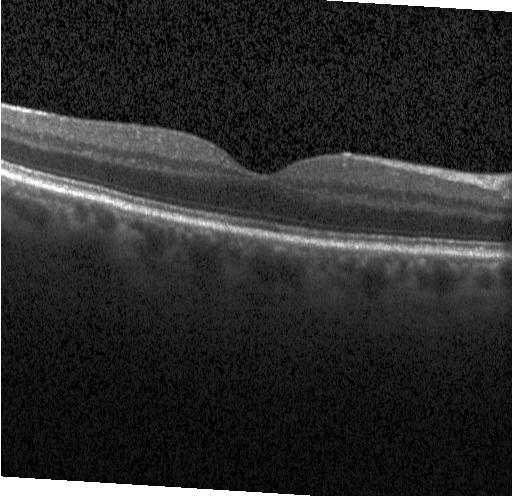
Dx: no choroidal neovascularization, diabetic macular edema, or drusen.